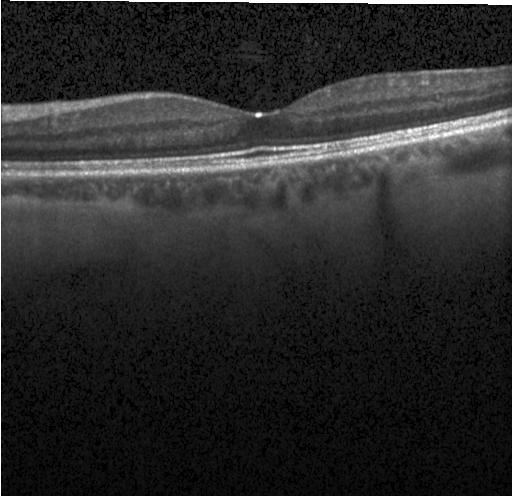

Finding: neither choroidal neovascularization, diabetic macular edema, nor drusen.